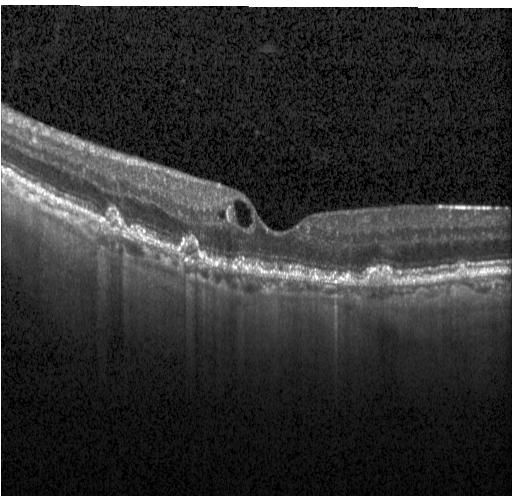
OCT line scan — A choroidal neovascular membrane.